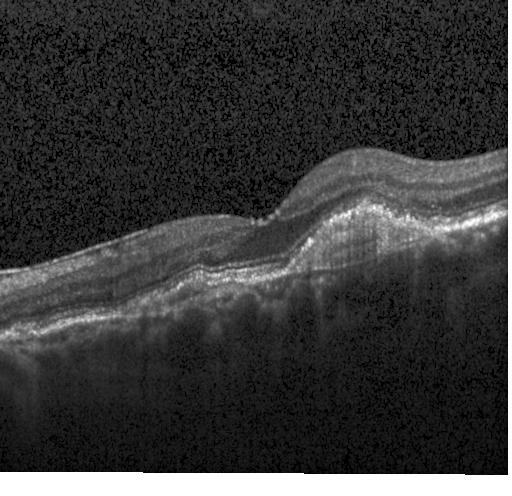
Dx: a choroidal neovascular membrane.